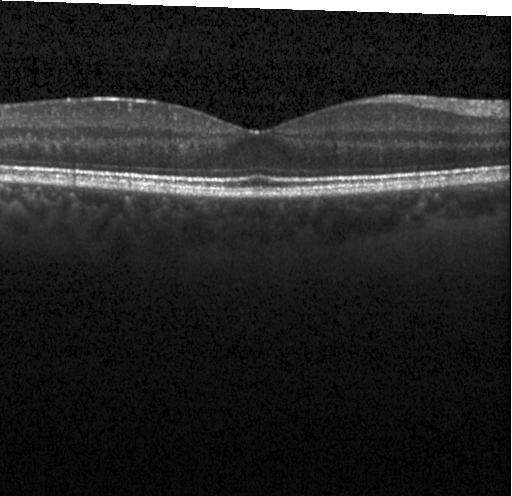 Retinal OCT cross-section · centered on the fovea · spectral-domain OCT · acquired on a Heidelberg Spectralis. Diagnosis: no choroidal neovascularization, no diabetic macular edema, and no drusen.